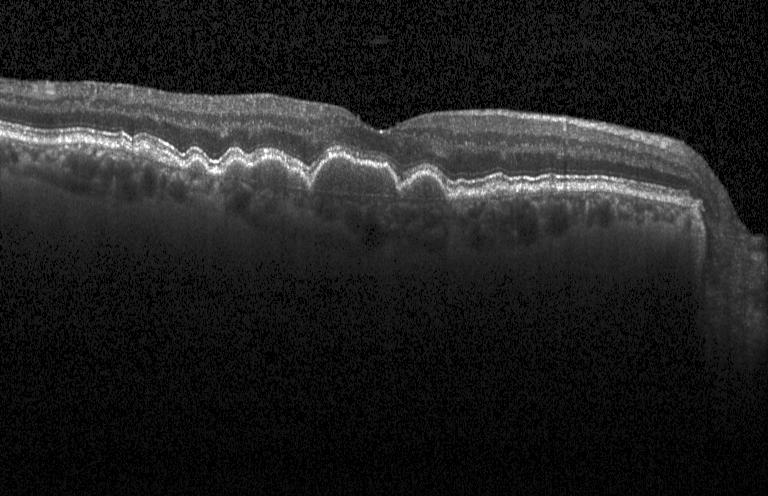 OCT line scan · spectral-domain OCT · instrument: Heidelberg Spectralis. OCT finding: multiple drusen.